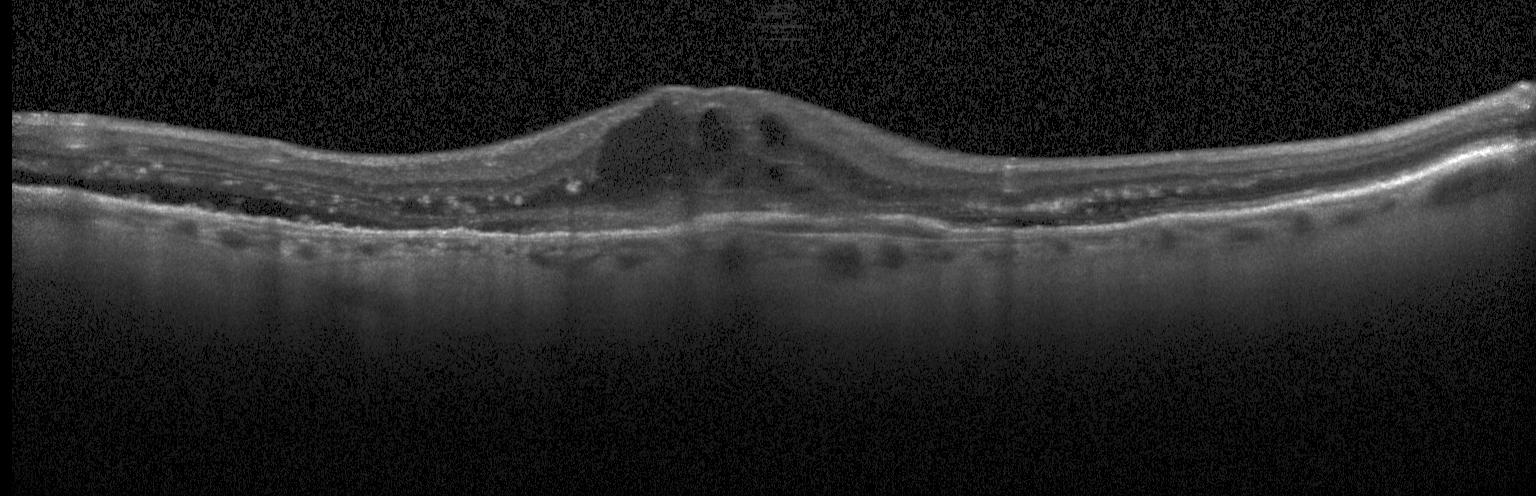

Macular OCT: a choroidal neovascular membrane.